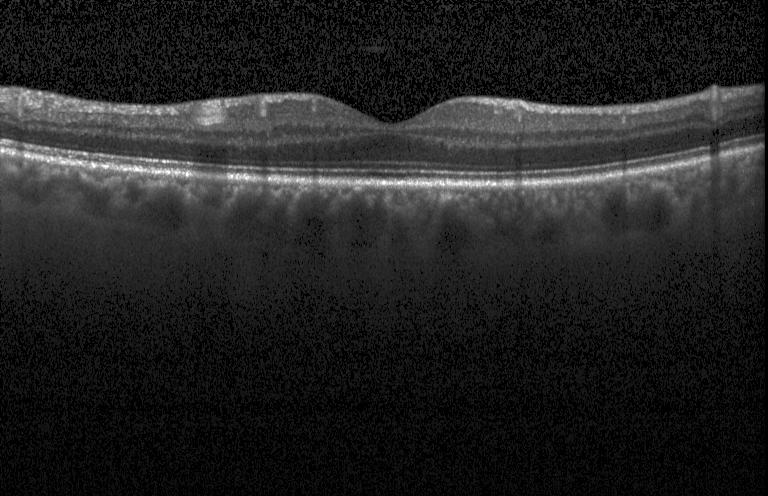

Heidelberg Spectralis OCT system. OCT line scan — This B-scan demonstrates no choroidal neovascularization, no diabetic macular edema, and no drusen.